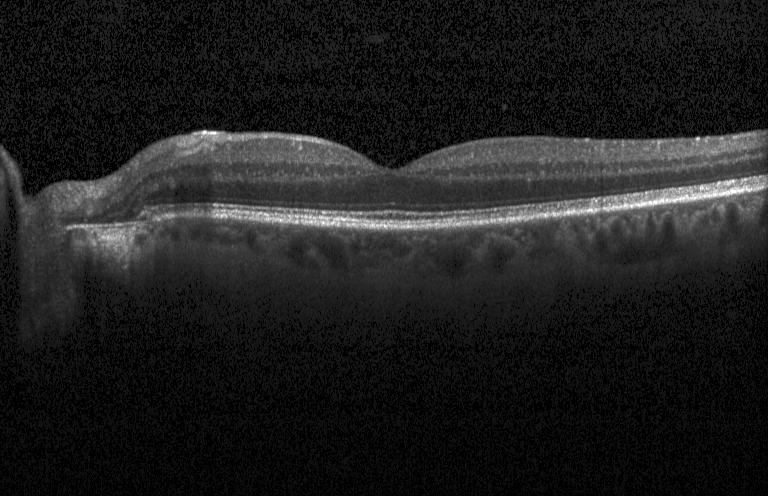 Optical coherence tomography scan. Spectral-domain optical coherence tomography.
Diagnosis: no CNV, DME, or drusen.